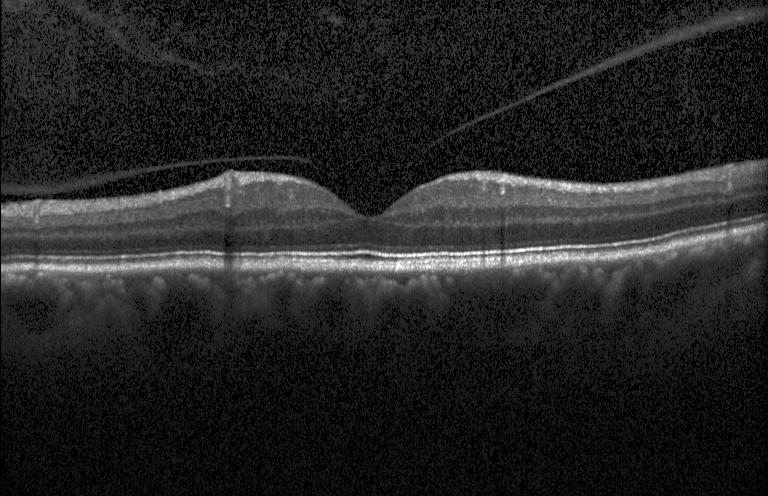 Retinal OCT B-scan, spectral-domain optical coherence tomography, horizontal scan through the fovea, Heidelberg Spectralis OCT system. This B-scan demonstrates neither choroidal neovascularization, diabetic macular edema, nor drusen.